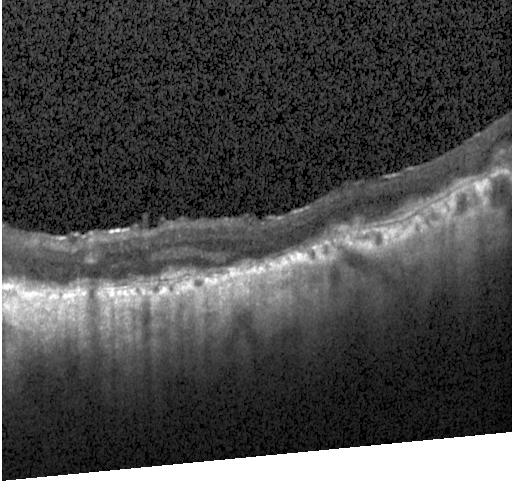
SD-OCT. Instrument: Heidelberg Spectralis. OCT B-scan
Dx: a choroidal neovascular membrane.